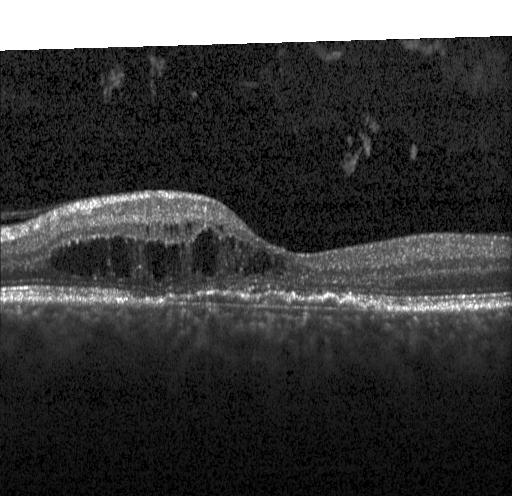 Impression: choroidal neovascularization.